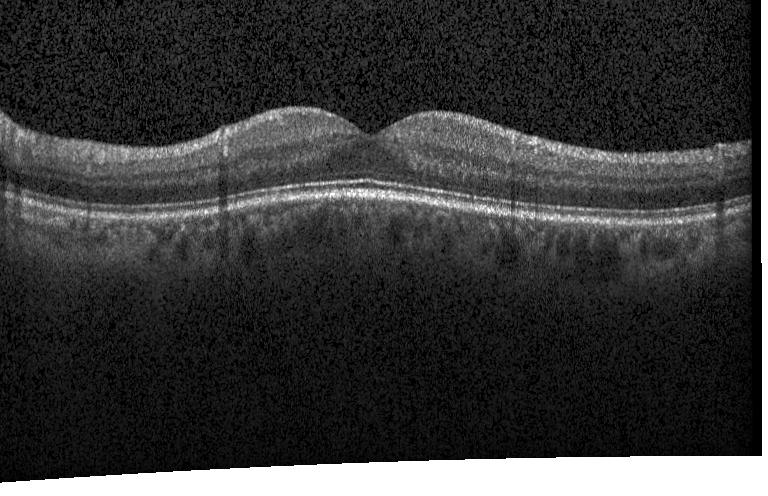 Instrument: Heidelberg Spectralis; spectral-domain OCT; OCT B-scan — Finding: no evidence of choroidal neovascularization, diabetic macular edema, or drusen.